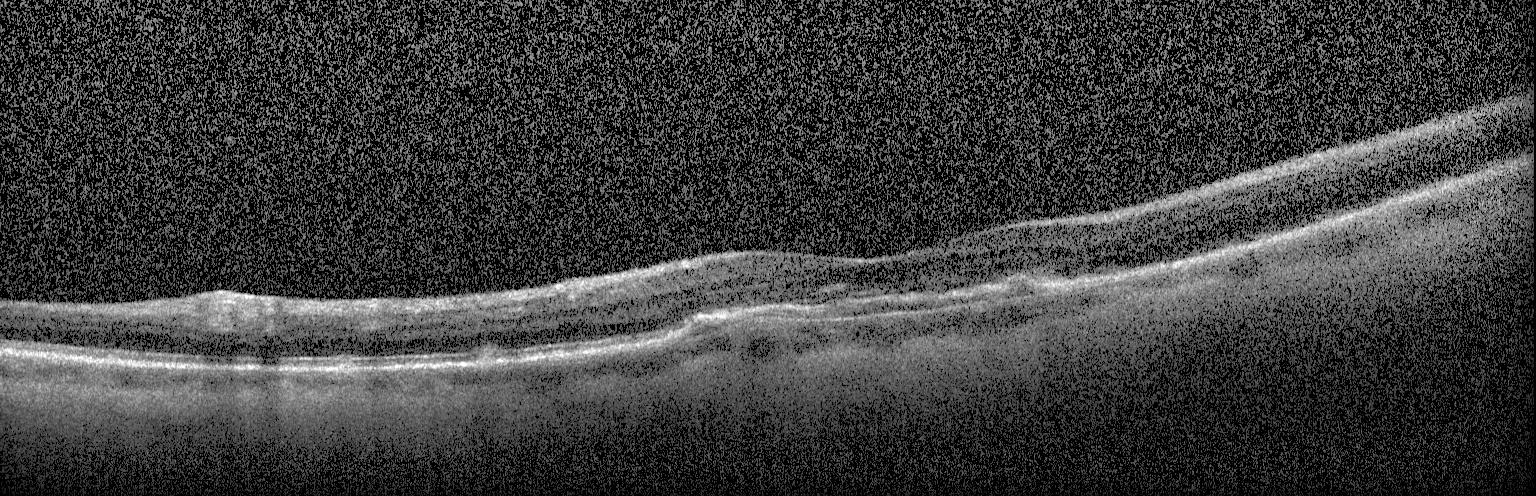

OCT line scan.
Impression: choroidal neovascularization.